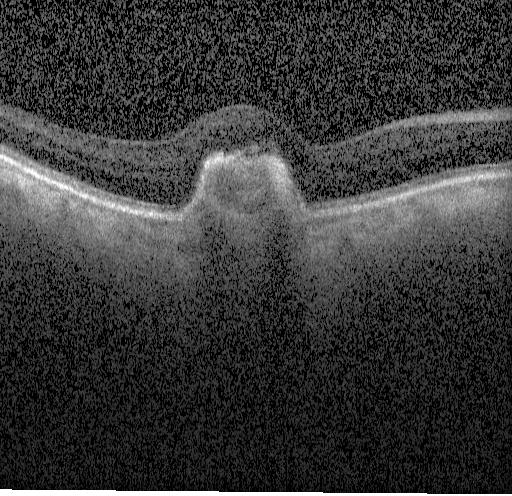 Retinal OCT cross-section
The scan shows a choroidal neovascular membrane.